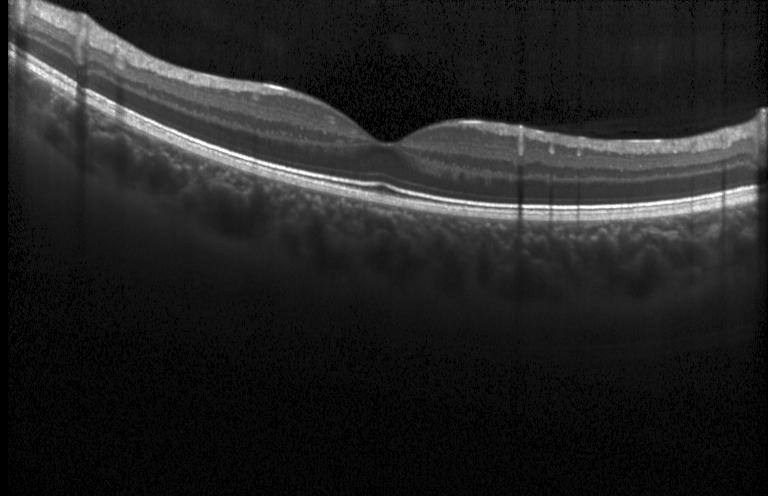
Heidelberg Spectralis OCT system, macular scan, OCT line scan, spectral-domain optical coherence tomography.
No evidence of choroidal neovascularization, diabetic macular edema, or drusen.